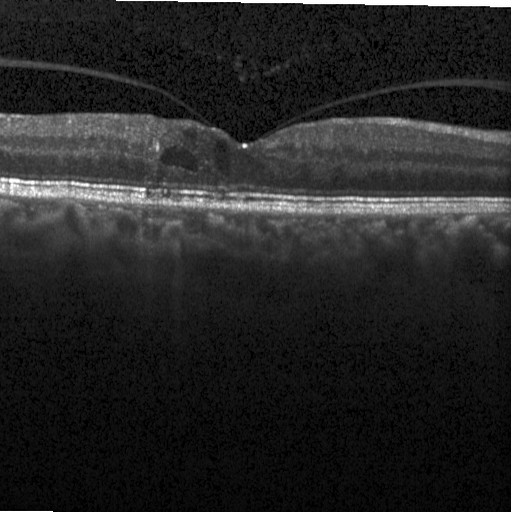
OCT B-scan showing DME.